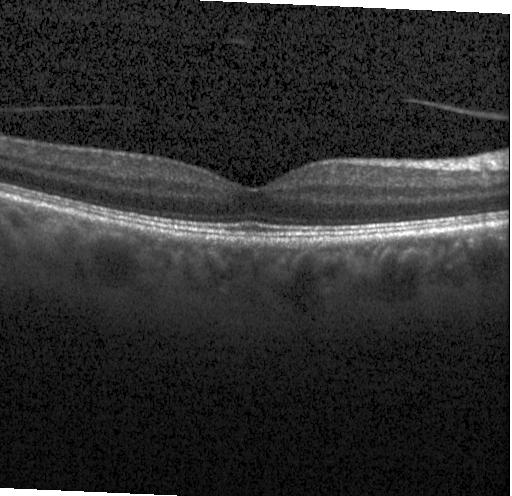
OCT scan showing neither CNV, DME, nor drusen.